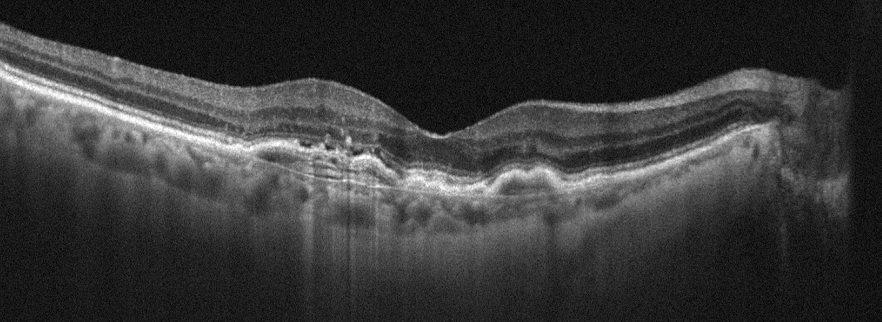

Optical coherence tomography B-scan · oculus dexter — Finding: age-related macular degeneration (AMD).